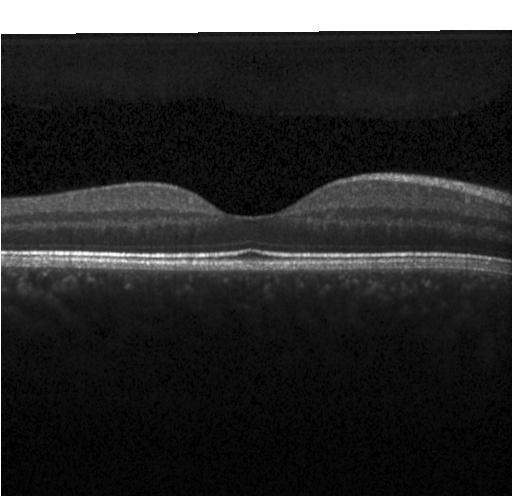

OCT B-scan. Macular scan. Acquired on a Heidelberg Spectralis. SD-OCT. Diagnosis: no choroidal neovascularization, no diabetic macular edema, and no drusen.